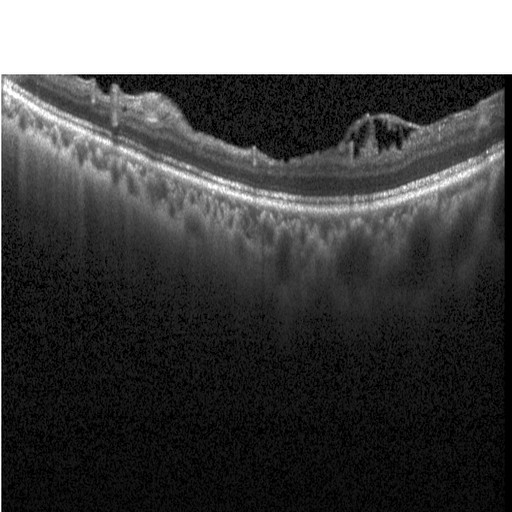 Acquired on a Heidelberg Spectralis, optical coherence tomography B-scan, spectral-domain OCT, through the macula.
Impression: diabetic macular edema (DME).